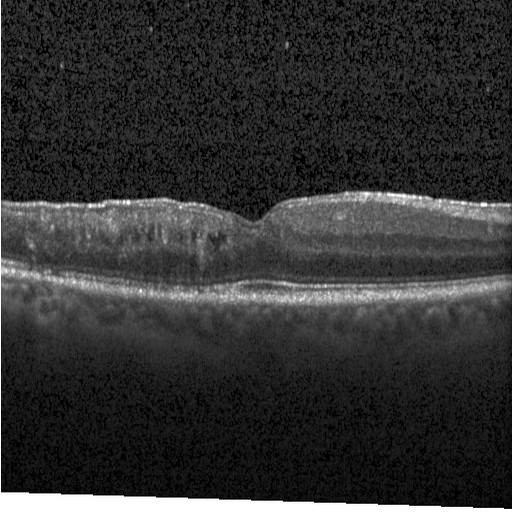 Retinal OCT B-scan, Heidelberg Spectralis OCT system — Assessment: DME.